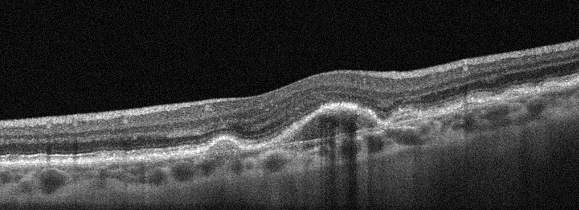 Retinal OCT cross-section; left eye; through the macula — Dx: age-related macular degeneration.